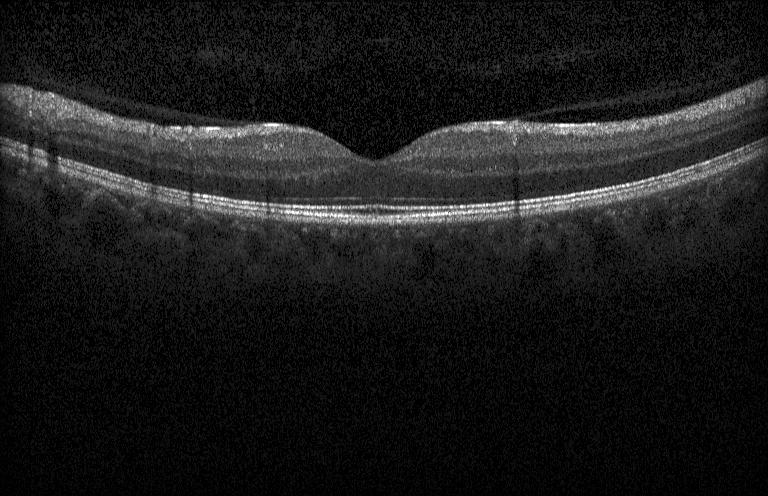
Retinal OCT B-scan
The scan shows no CNV, DME, or drusen.